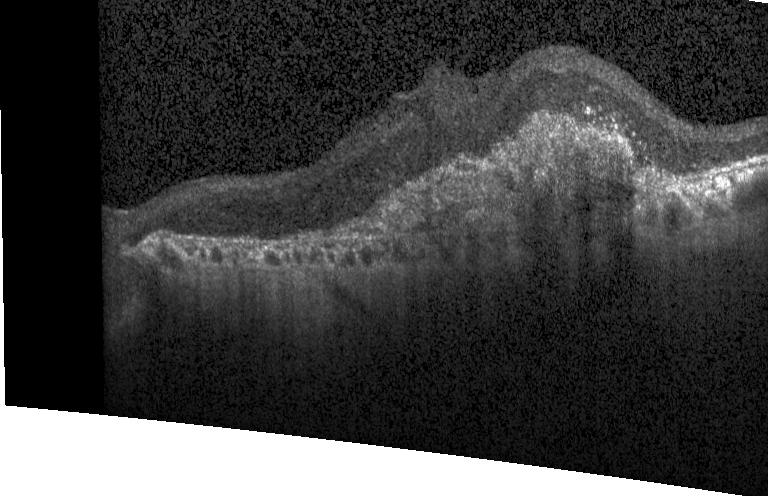 Impression: choroidal neovascularization (CNV).